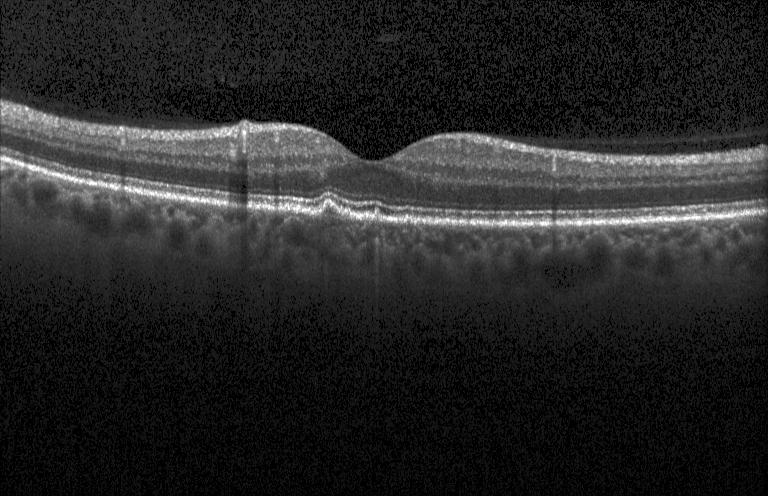
Macular OCT: multiple drusen.